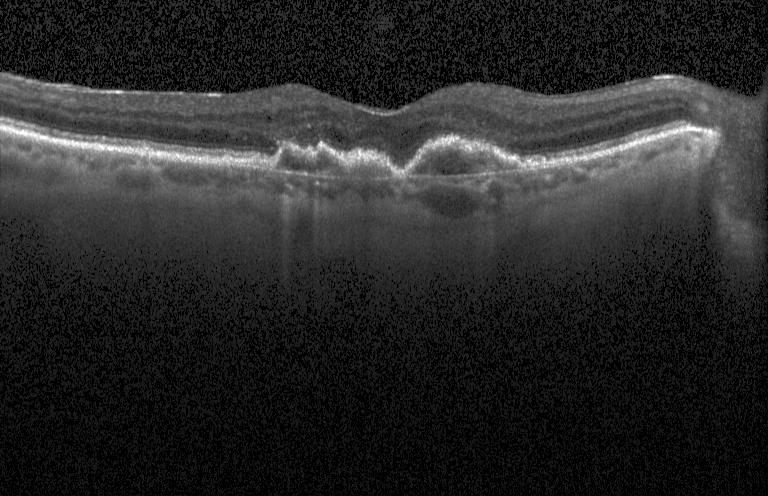
Spectral-domain OCT. Heidelberg Spectralis. Optical coherence tomography scan. Centered on the fovea
Dx: a choroidal neovascular membrane.